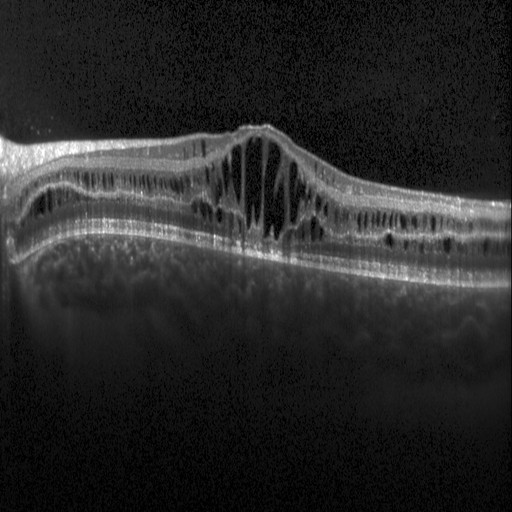
Retinal OCT cross-section. Dx: diabetic macular edema.